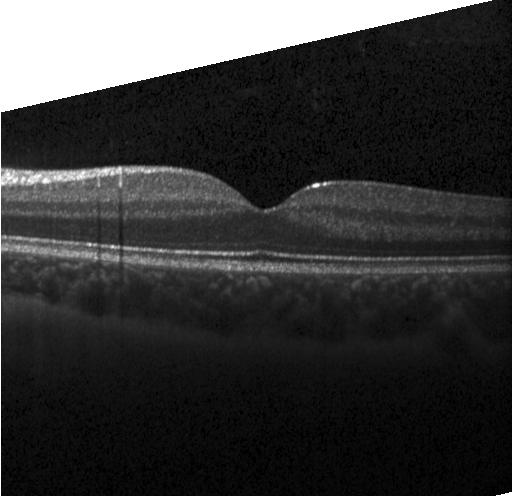

Macular OCT: neither choroidal neovascularization, diabetic macular edema, nor drusen.